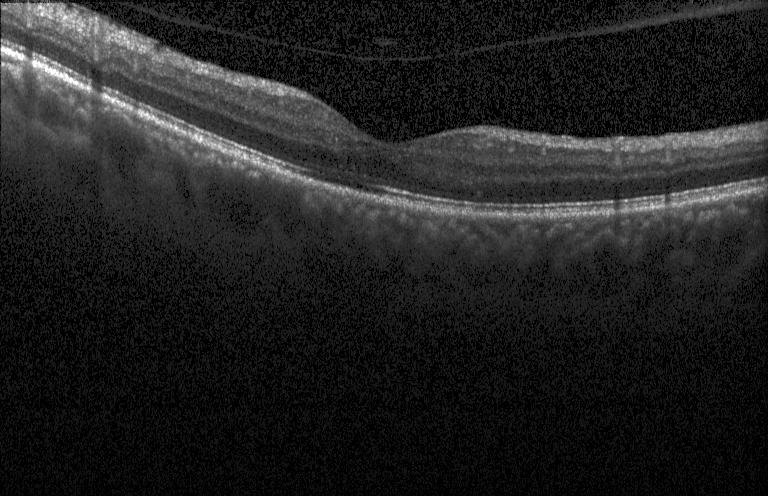 Macular OCT: no choroidal neovascularization, no diabetic macular edema, and no drusen.